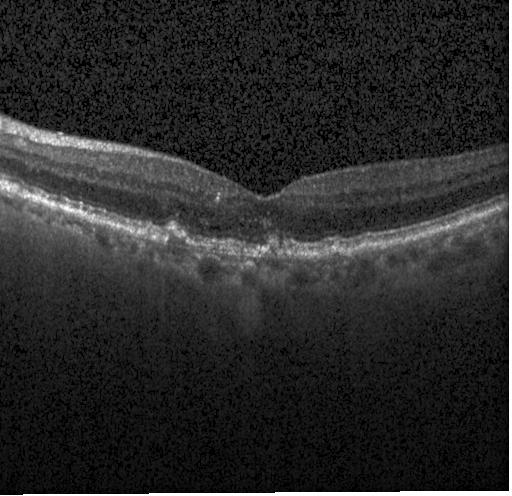 Fovea-centered, optical coherence tomography scan, spectral-domain OCT, instrument: Heidelberg Spectralis — Impression: sub-RPE drusenoid deposits.